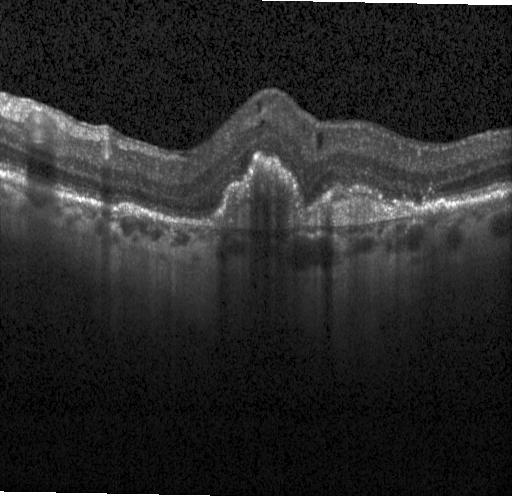

OCT scan showing a choroidal neovascular membrane.